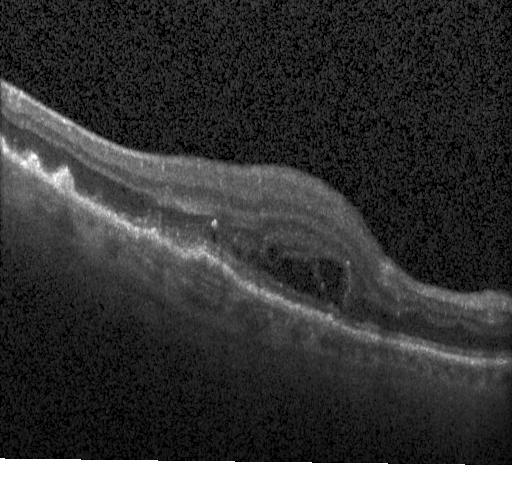
Retinal OCT cross-section · Heidelberg Spectralis · centered on the fovea · spectral-domain optical coherence tomography — Diagnosis: a choroidal neovascular membrane.